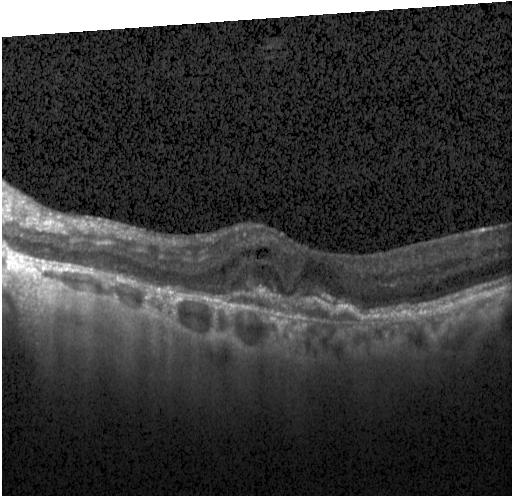
Spectral-domain OCT B-scan: a choroidal neovascular membrane.